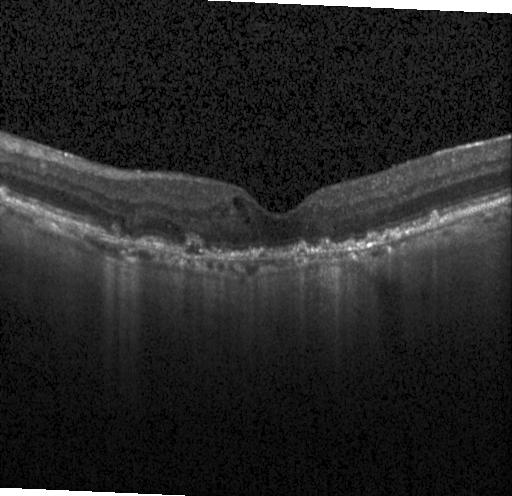 A choroidal neovascular membrane.